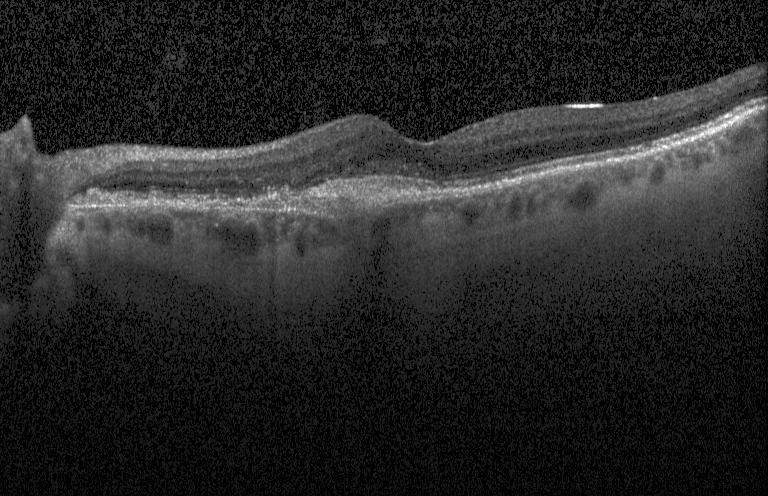
OCT B-scan, spectral-domain optical coherence tomography. CNV.